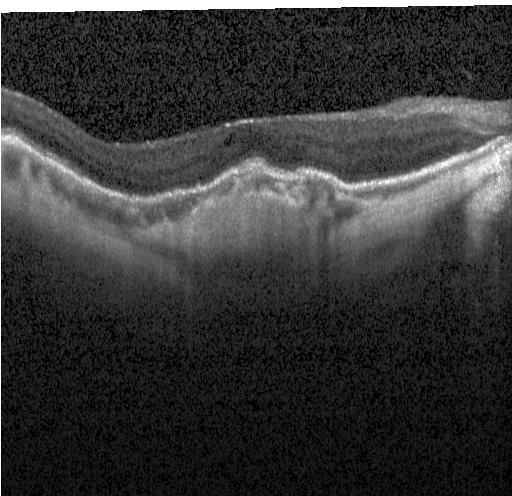
Diagnosis: a choroidal neovascular membrane.